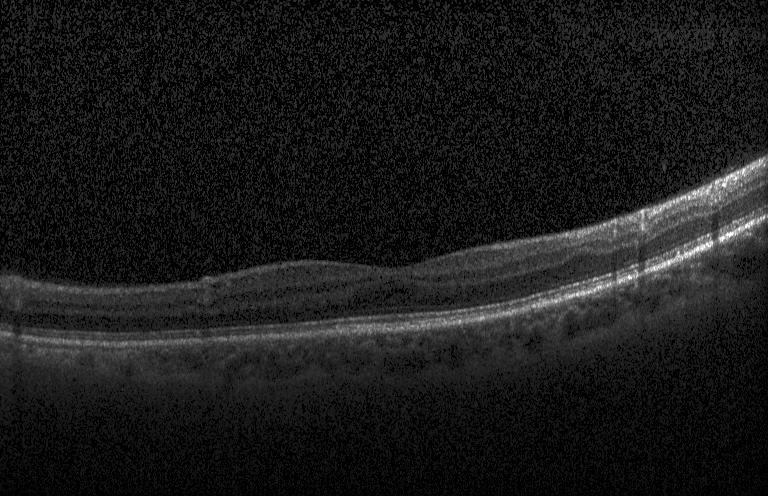

Optical coherence tomography scan
The scan shows no choroidal neovascularization, no diabetic macular edema, and no drusen.